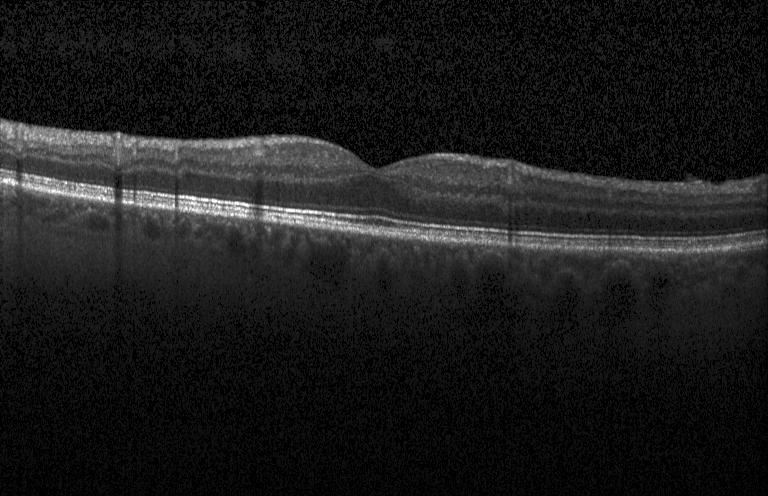 Macular OCT: no CNV, no DME, and no drusen.